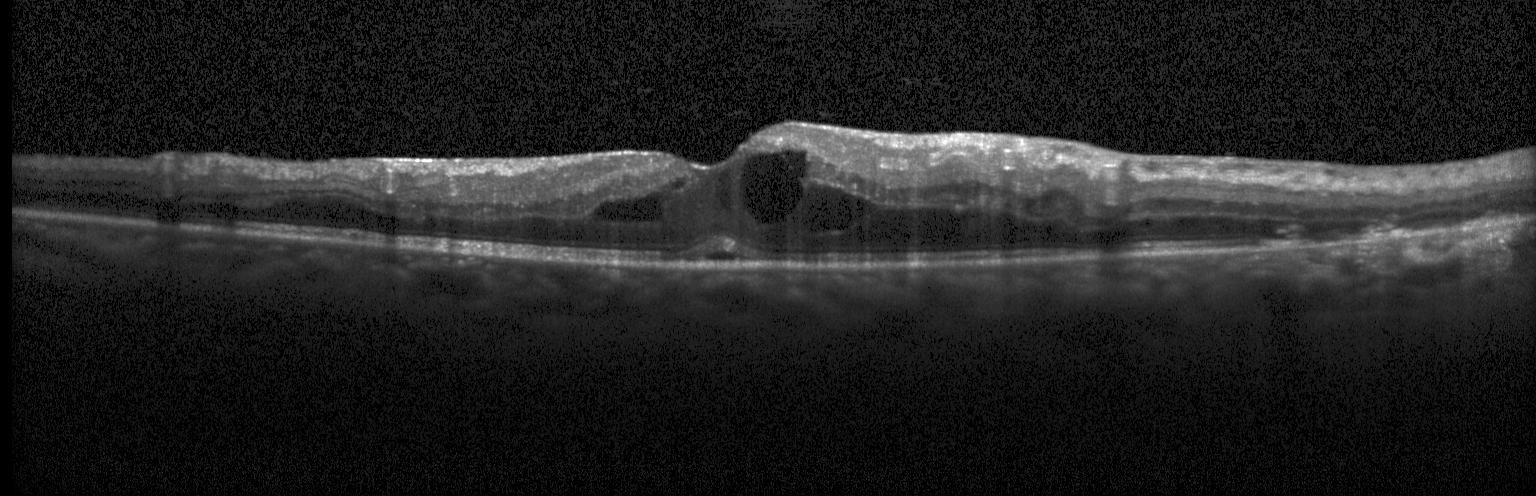

Dx: diabetic macular edema (DME).